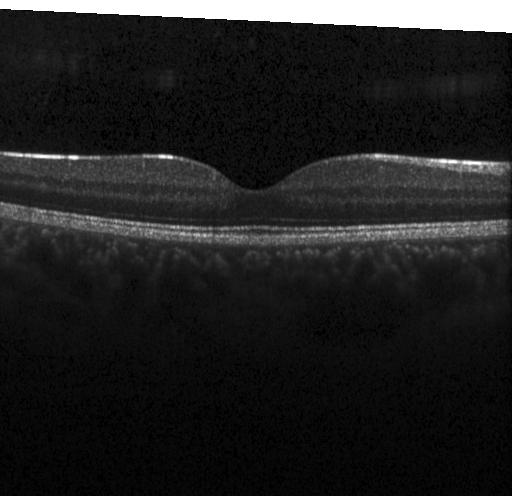 SD-OCT. Horizontal scan through the fovea. OCT line scan.
Diagnosis: no evidence of choroidal neovascularization, diabetic macular edema, or drusen.